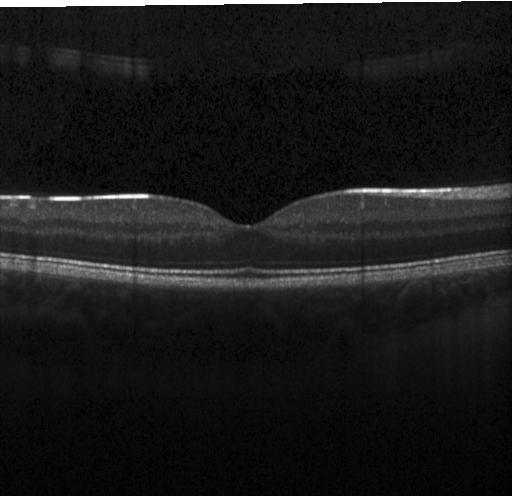
Optical coherence tomography scan, centered on the fovea.
Assessment: no choroidal neovascularization, no diabetic macular edema, and no drusen.